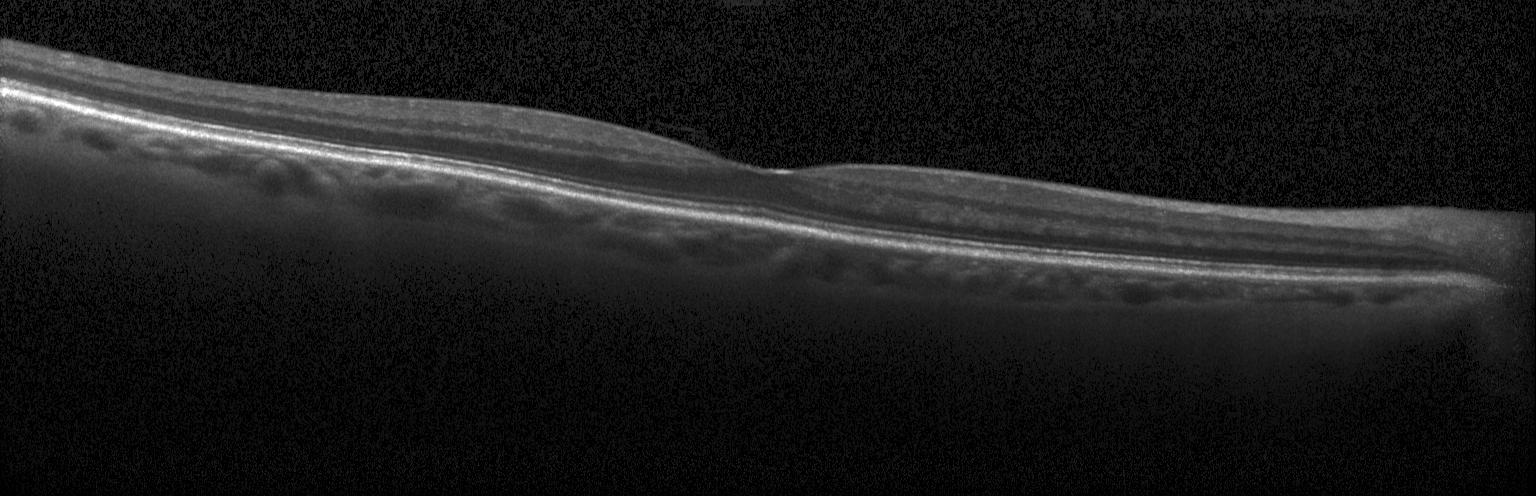

Impression: no choroidal neovascularization, diabetic macular edema, or drusen.